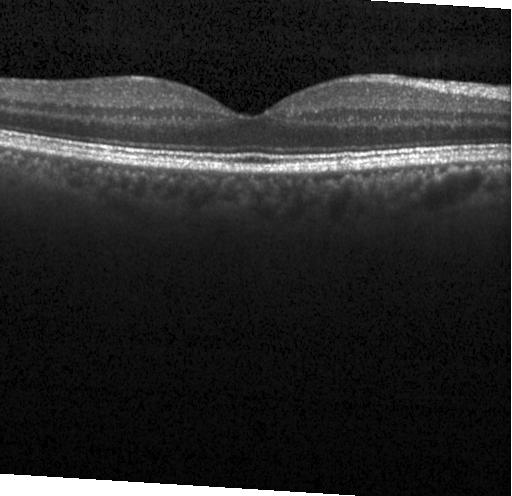

No choroidal neovascularization, diabetic macular edema, or drusen.